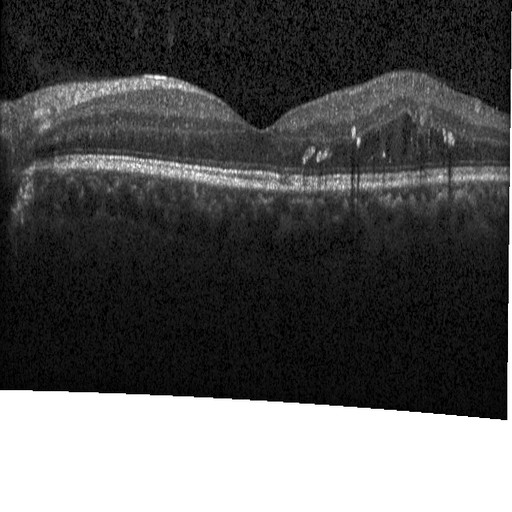

Spectral-domain OCT B-scan: diabetic macular edema (DME).